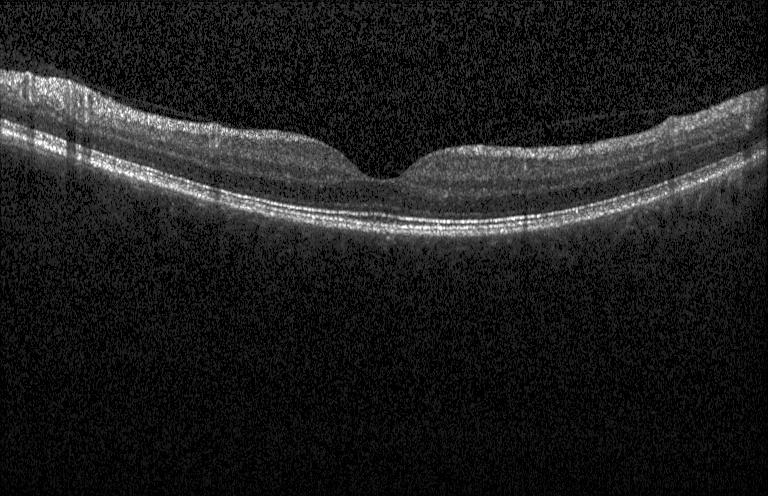
Optical coherence tomography B-scan. Macular scan — Macular OCT: no choroidal neovascularization, no diabetic macular edema, and no drusen.